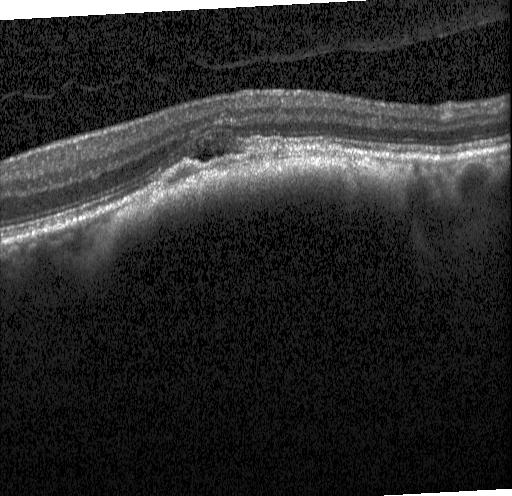 Acquired on a Heidelberg Spectralis, SD-OCT, optical coherence tomography B-scan
Diagnosis: CNV.